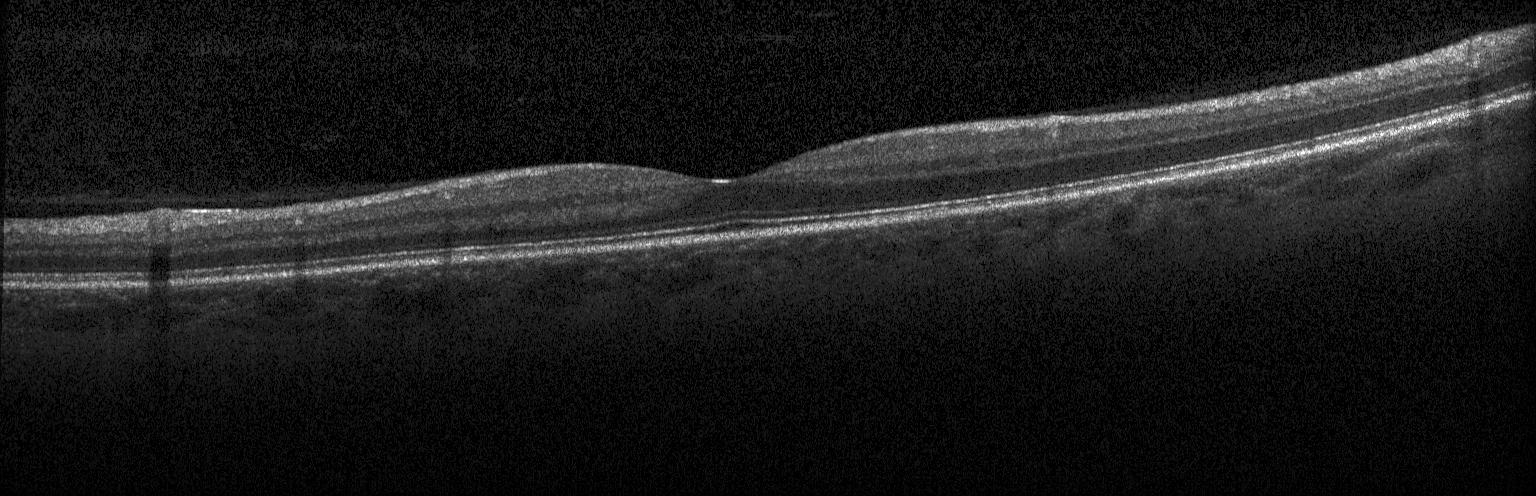 Horizontal scan through the fovea, acquired on a Heidelberg Spectralis, spectral-domain OCT, optical coherence tomography scan. Assessment: no CNV, no DME, and no drusen.